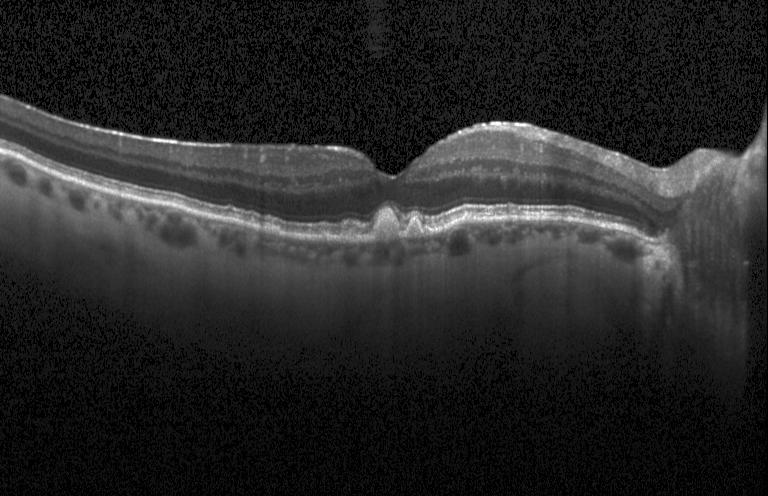
SD-OCT, macular scan, OCT line scan. Macular OCT: multiple drusen.